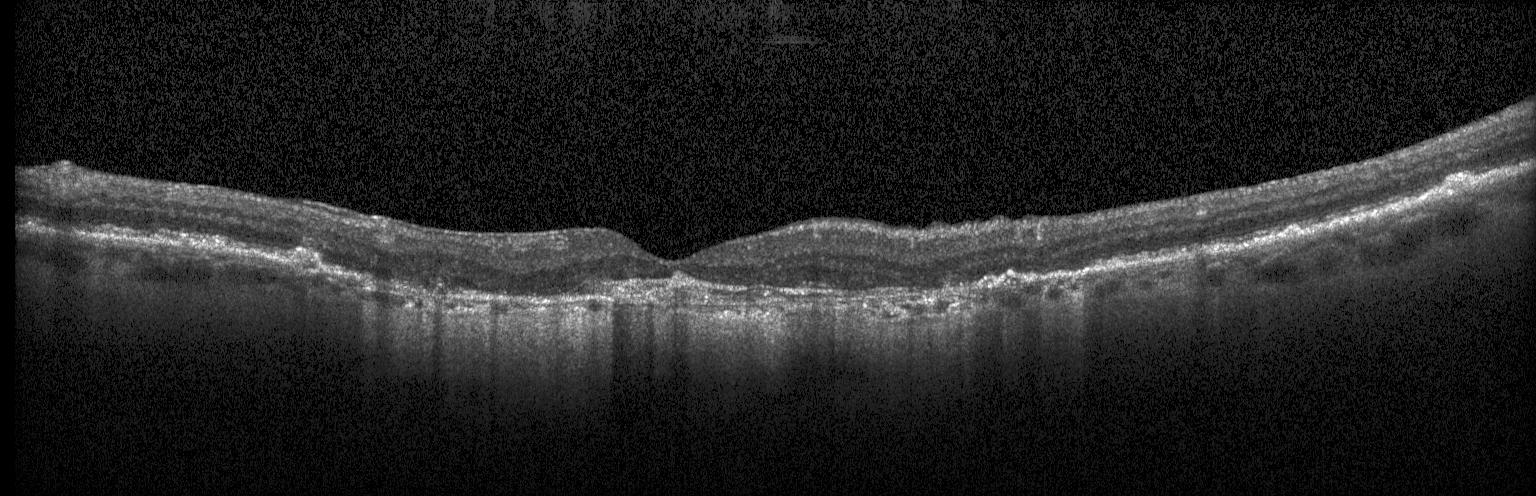
Finding: a choroidal neovascular membrane.